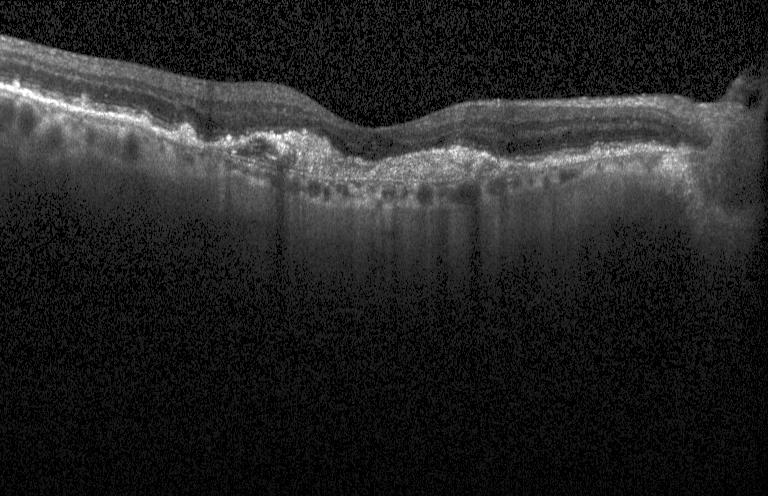
Heidelberg Spectralis; OCT line scan; centered on the fovea; spectral-domain optical coherence tomography. Macular OCT: choroidal neovascularization (CNV).